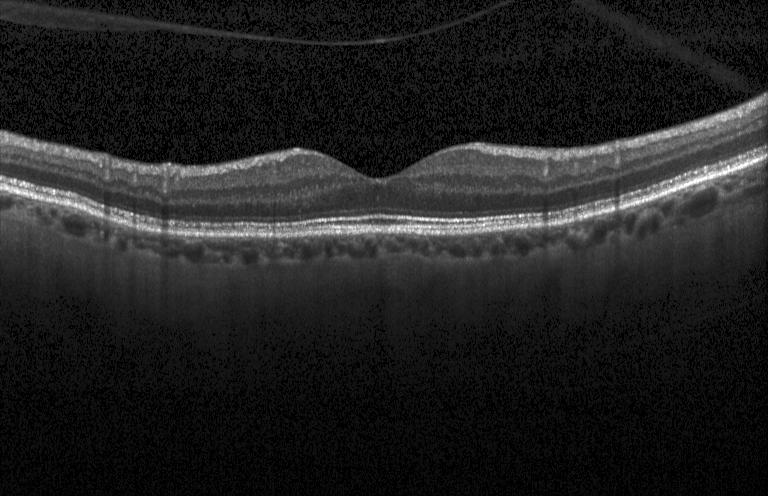 Acquired on a Heidelberg Spectralis, SD-OCT, retinal OCT B-scan — Finding: neither choroidal neovascularization, diabetic macular edema, nor drusen.